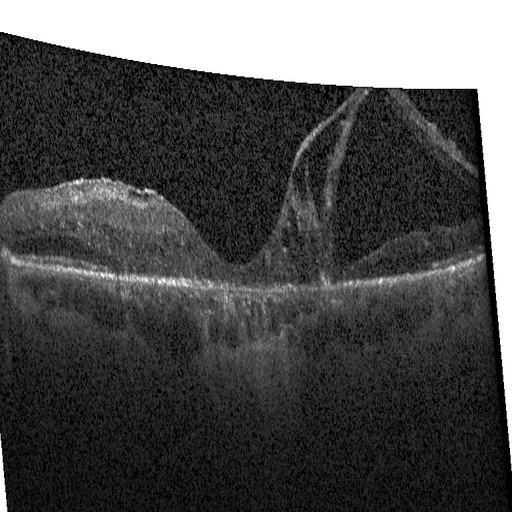

Finding: DME.